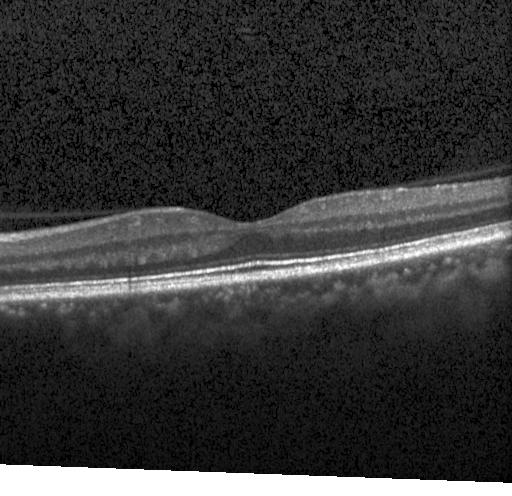 Dx: no evidence of choroidal neovascularization, diabetic macular edema, or drusen.